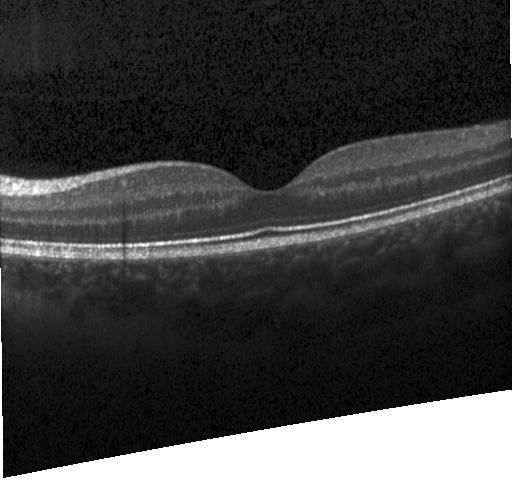

Dx: no choroidal neovascularization, no diabetic macular edema, and no drusen.